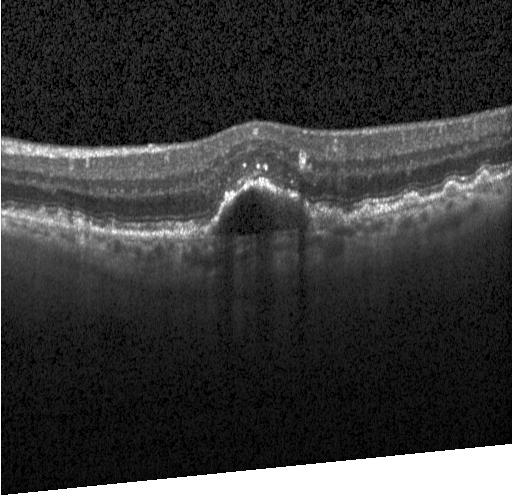 The scan shows a choroidal neovascular membrane.